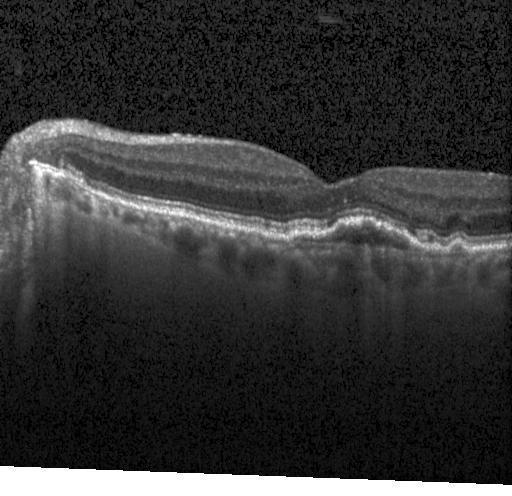

Diagnosis: a choroidal neovascular membrane.